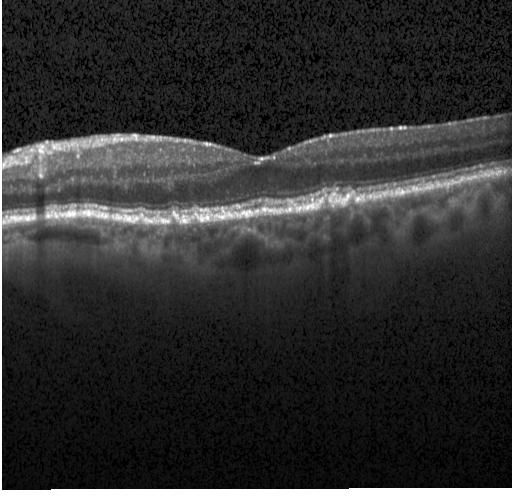

Finding: multiple drusen.